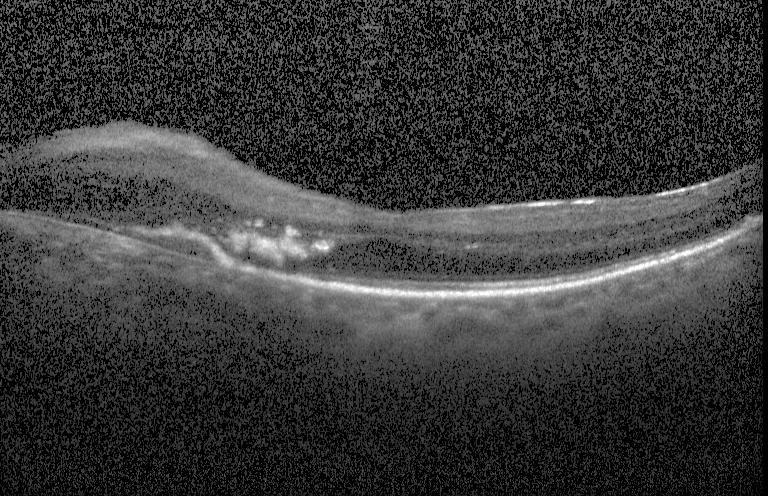

Optical coherence tomography scan; spectral-domain OCT. Impression: choroidal neovascularization.